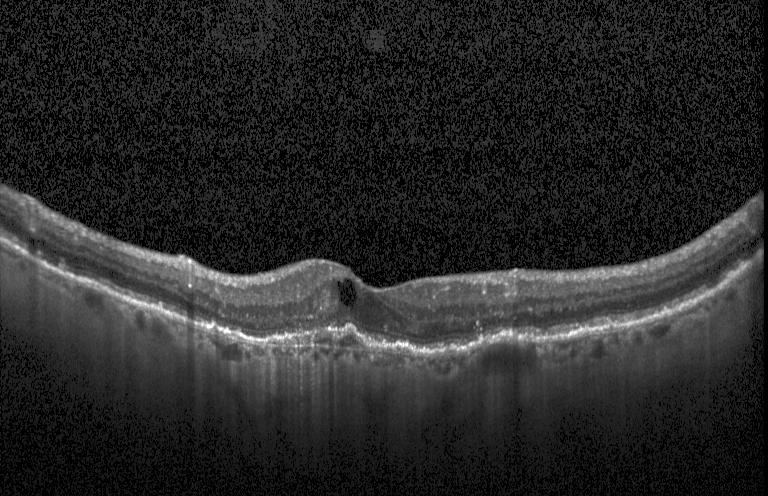

The scan shows a choroidal neovascular membrane.